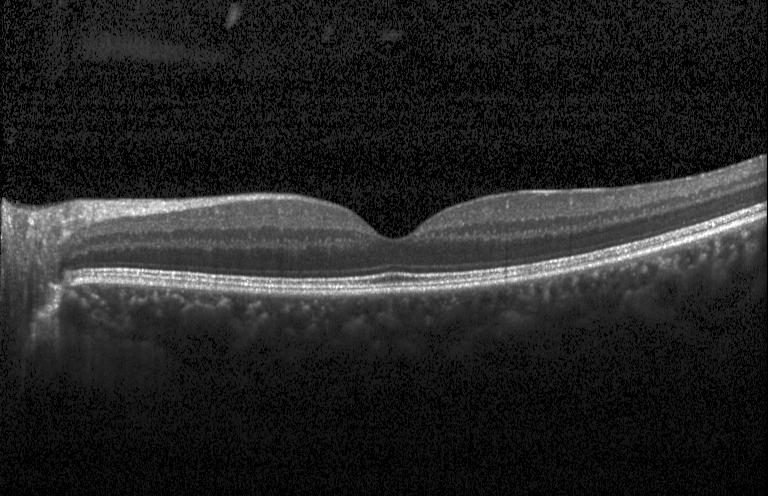 Optical coherence tomography B-scan, centered on the fovea
Impression: no CNV, DME, or drusen.